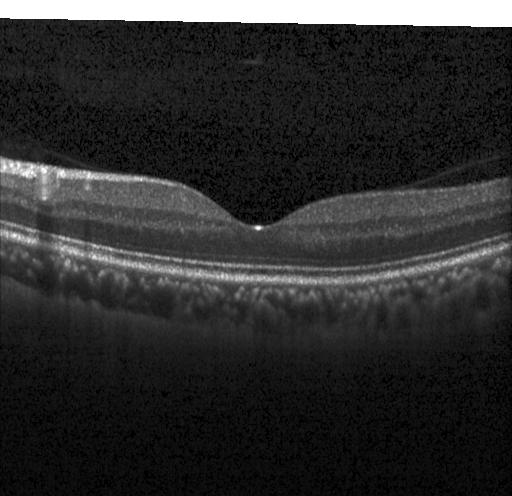

Fovea-centered. OCT line scan. Diagnosis: neither choroidal neovascularization, diabetic macular edema, nor drusen.